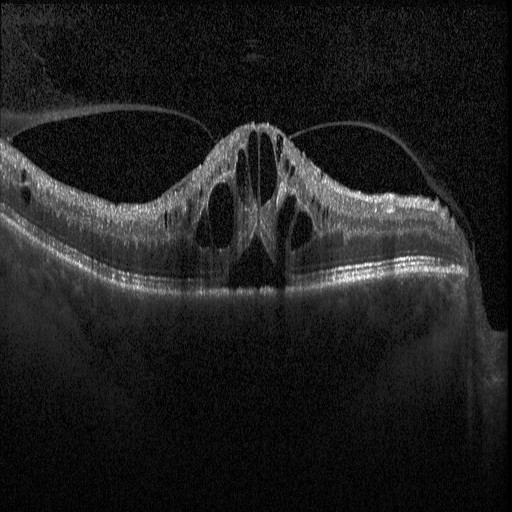 Diabetic macular edema (DME).